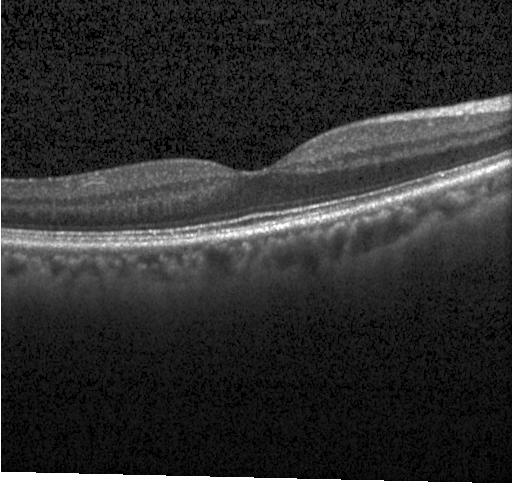

Retinal OCT cross-section. The scan shows no evidence of choroidal neovascularization, diabetic macular edema, or drusen.